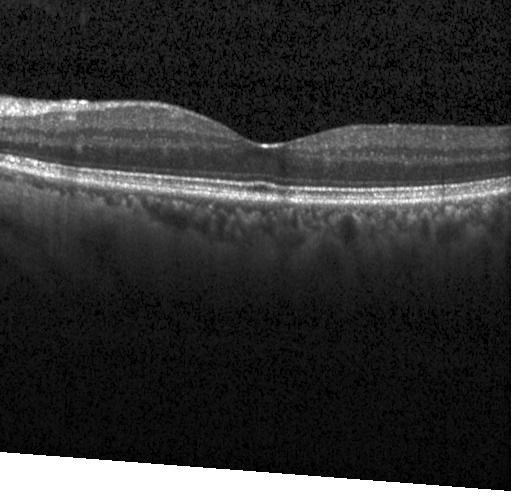
OCT line scan — Assessment: no CNV, no DME, and no drusen.